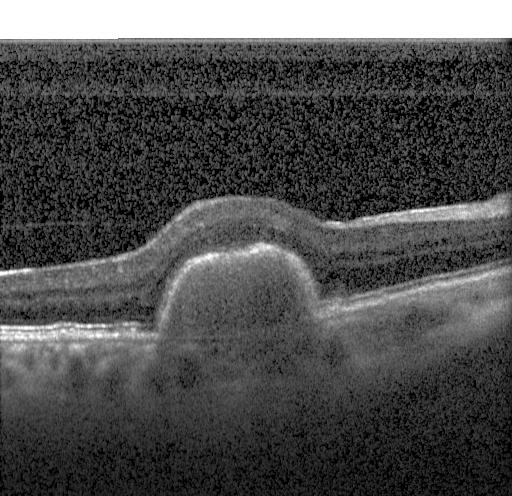
Spectral-domain OCT, through the macula, optical coherence tomography B-scan.
Choroidal neovascularization (CNV).